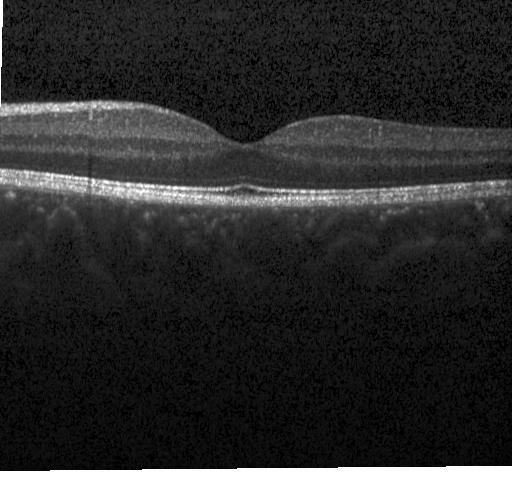

Through the macula; instrument: Heidelberg Spectralis; OCT B-scan; spectral-domain optical coherence tomography — Diagnosis: neither choroidal neovascularization, diabetic macular edema, nor drusen.